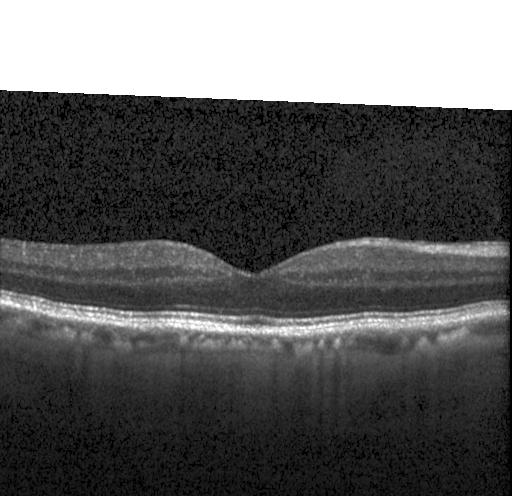
OCT line scan. Impression: no choroidal neovascularization, diabetic macular edema, or drusen.